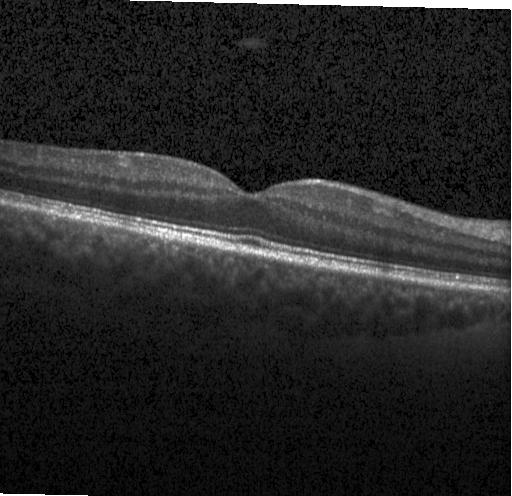 Finding: no CNV, DME, or drusen.